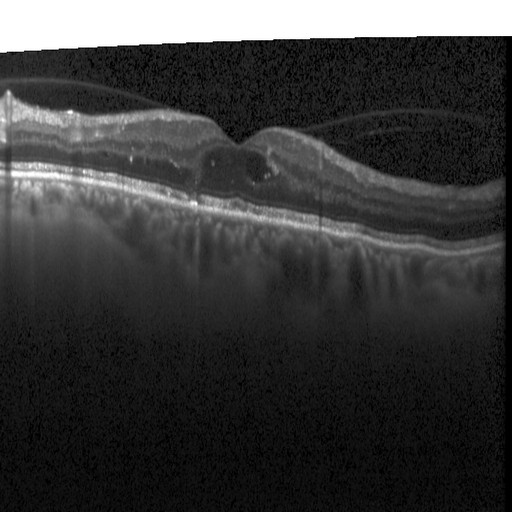

Optical coherence tomography scan. Macular OCT: DME.